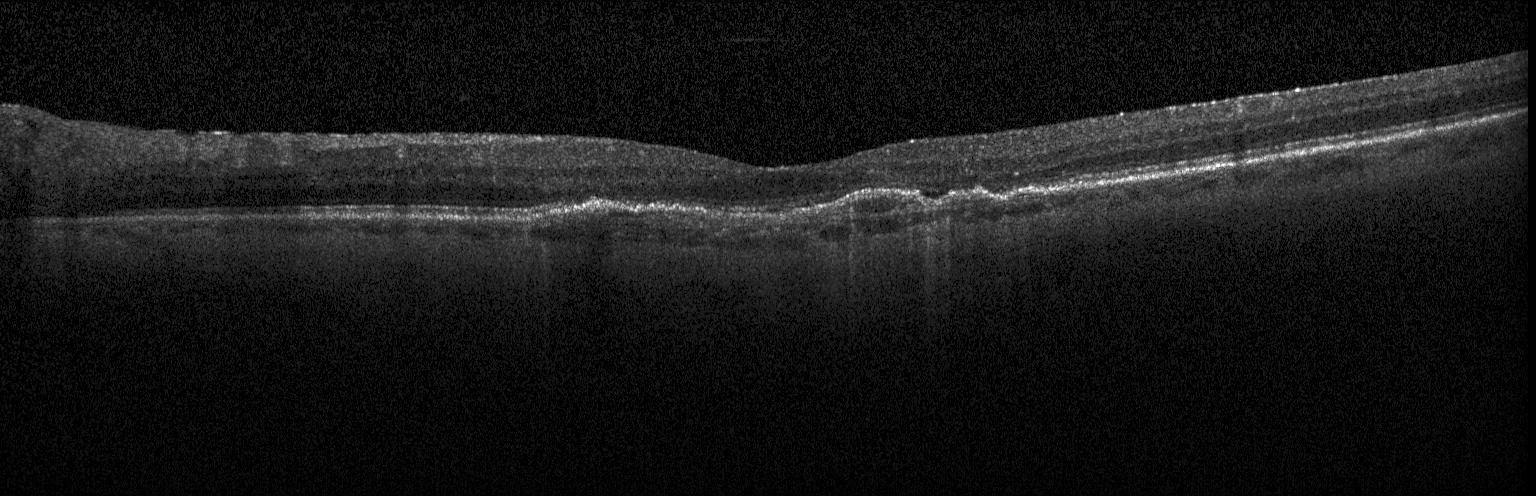
OCT finding: a choroidal neovascular membrane.